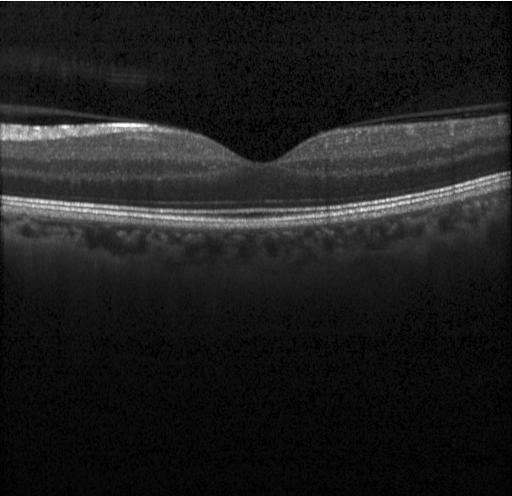

Retinal OCT cross-section showing no evidence of CNV, DME, or drusen.